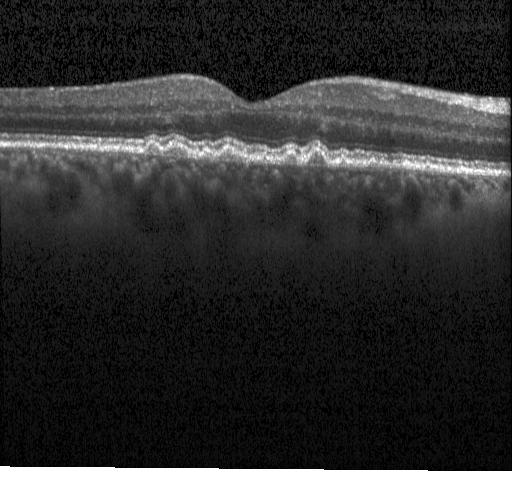
Through the macula · spectral-domain optical coherence tomography · OCT B-scan · instrument: Heidelberg Spectralis. Dx: sub-RPE drusenoid deposits.